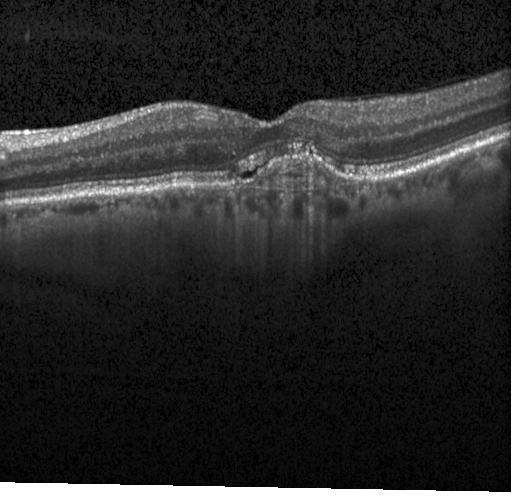
Spectral-domain OCT B-scan: a choroidal neovascular membrane.